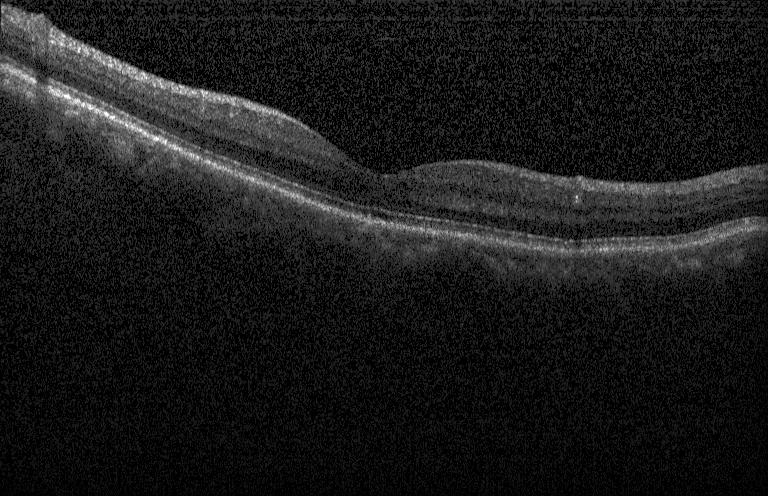
Centered on the fovea · spectral-domain OCT · retinal OCT B-scan · acquired on a Heidelberg Spectralis.
Assessment: neither choroidal neovascularization, diabetic macular edema, nor drusen.